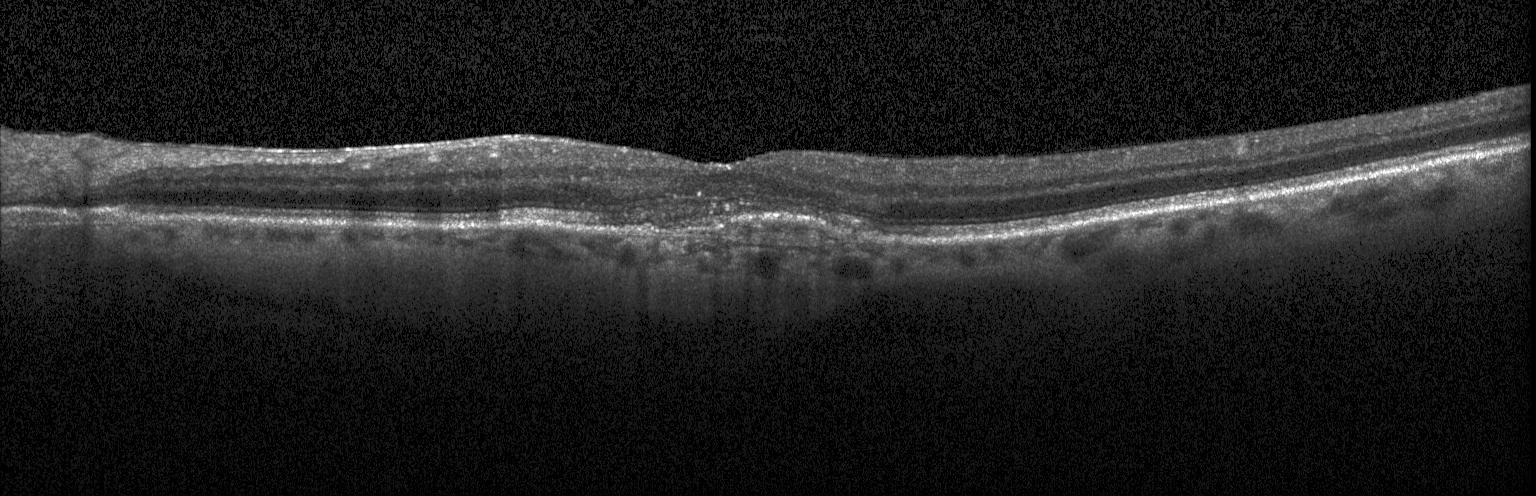 Optical coherence tomography B-scan
Dx: a choroidal neovascular membrane.